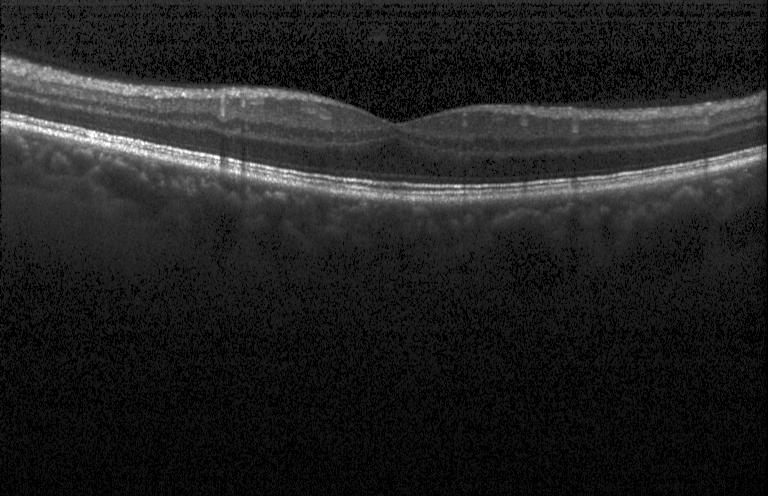 OCT line scan
Dx: no evidence of CNV, DME, or drusen.